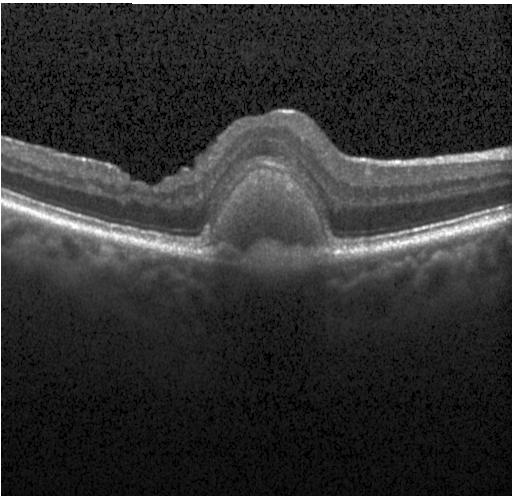

Heidelberg Spectralis, optical coherence tomography scan — The scan shows choroidal neovascularization.